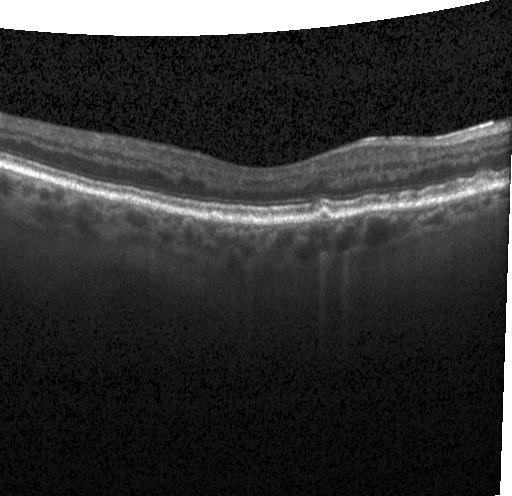 Macular OCT demonstrating multiple drusen.